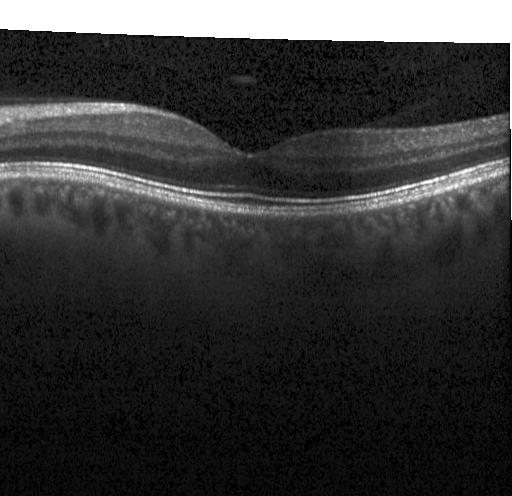 SD-OCT. Horizontal scan through the fovea. Acquired on a Heidelberg Spectralis. OCT B-scan — Finding: no choroidal neovascularization, no diabetic macular edema, and no drusen.